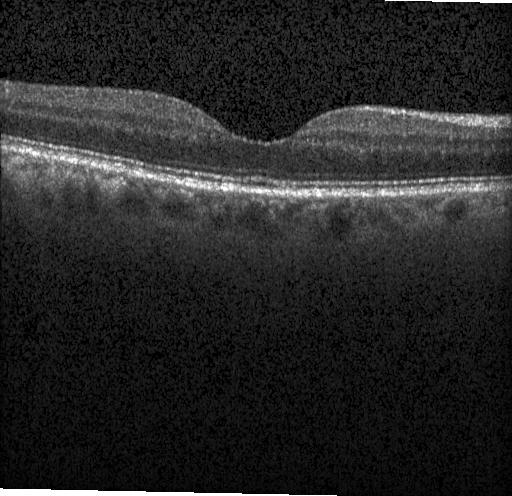
Horizontal scan through the fovea · acquired on a Heidelberg Spectralis · optical coherence tomography B-scan — No choroidal neovascularization, diabetic macular edema, or drusen.